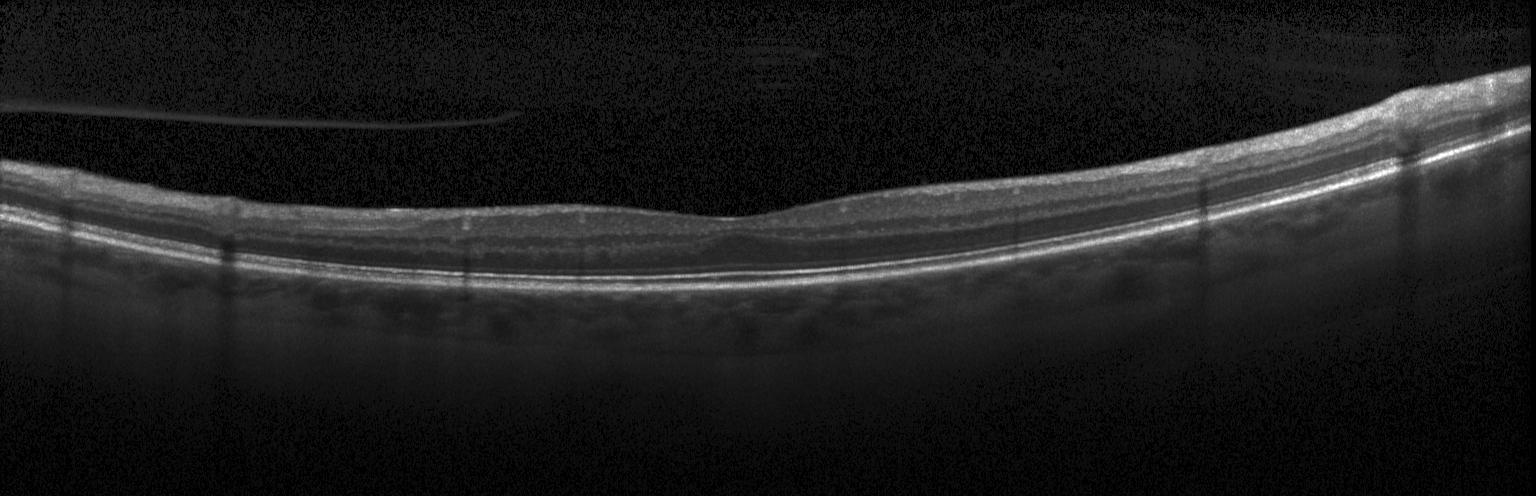
Retinal OCT cross-section showing neither choroidal neovascularization, diabetic macular edema, nor drusen.